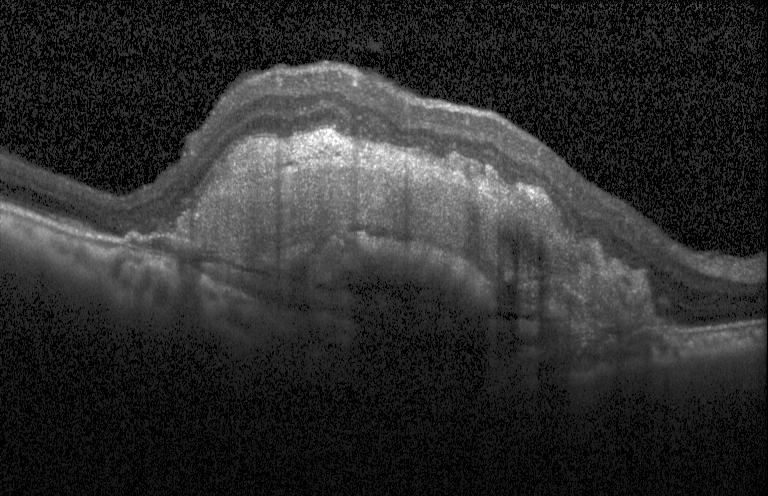
Assessment: a choroidal neovascular membrane.